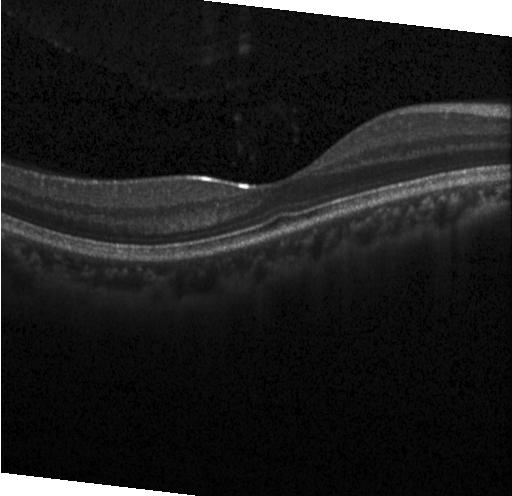 Impression: no evidence of choroidal neovascularization, diabetic macular edema, or drusen.